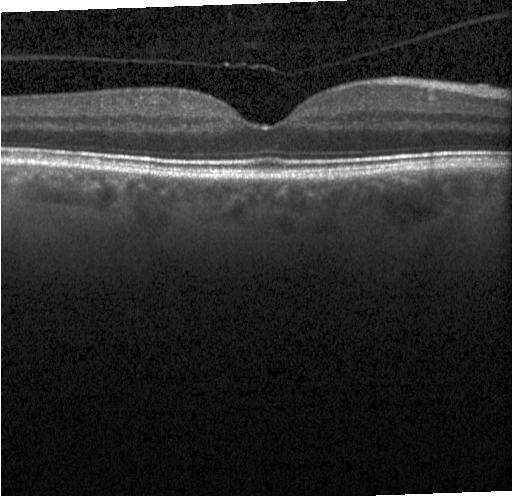

Retinal OCT cross-section, instrument: Heidelberg Spectralis — Assessment: no evidence of choroidal neovascularization, diabetic macular edema, or drusen.